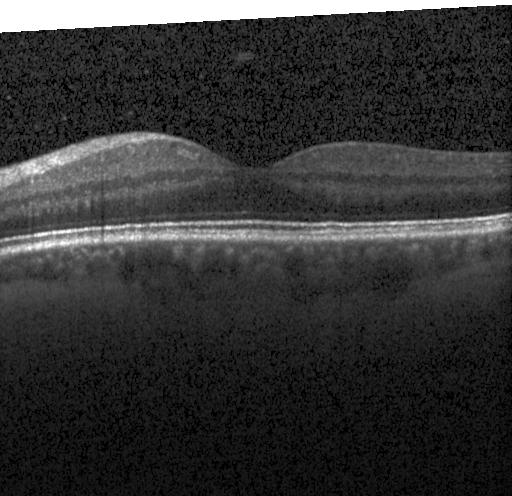 Assessment: no choroidal neovascularization, no diabetic macular edema, and no drusen.